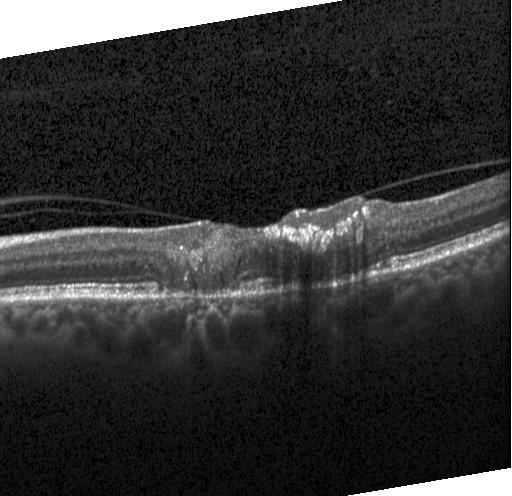

Acquired on a Heidelberg Spectralis; OCT B-scan; spectral-domain OCT.
The scan shows choroidal neovascularization (CNV).